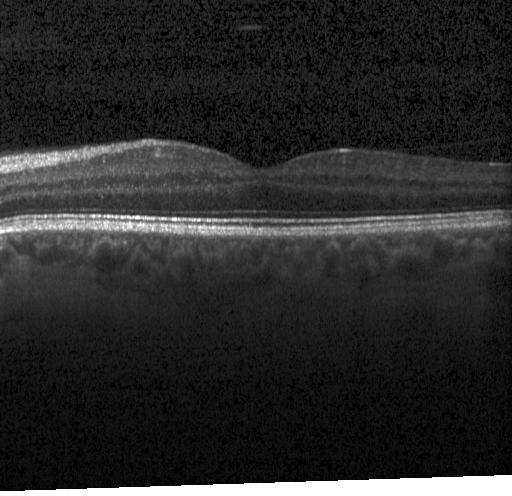
Retinal OCT cross-section
Impression: no choroidal neovascularization, diabetic macular edema, or drusen.